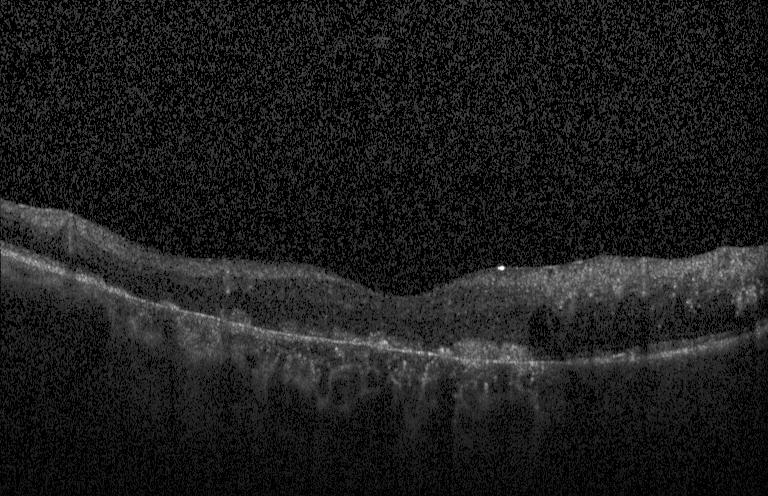 Macular OCT: CNV.